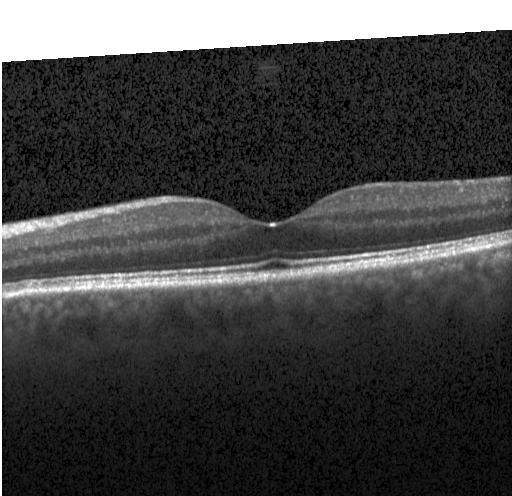
Spectral-domain OCT B-scan: neither choroidal neovascularization, diabetic macular edema, nor drusen.